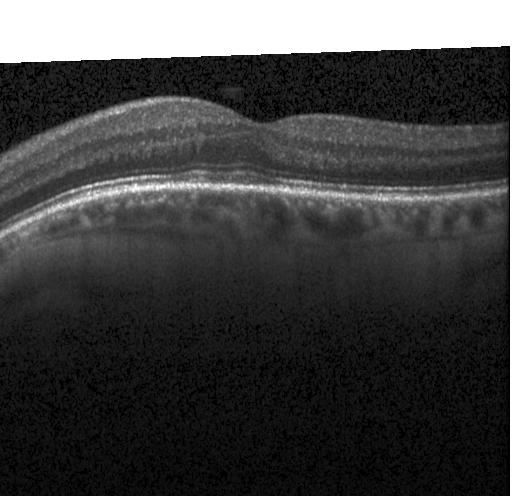 Optical coherence tomography scan.
Finding: no choroidal neovascularization, no diabetic macular edema, and no drusen.